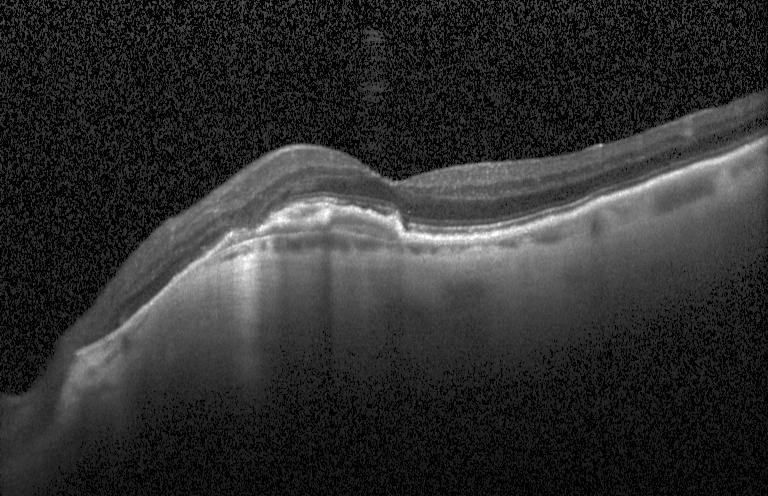

OCT B-scan — The scan shows a choroidal neovascular membrane.